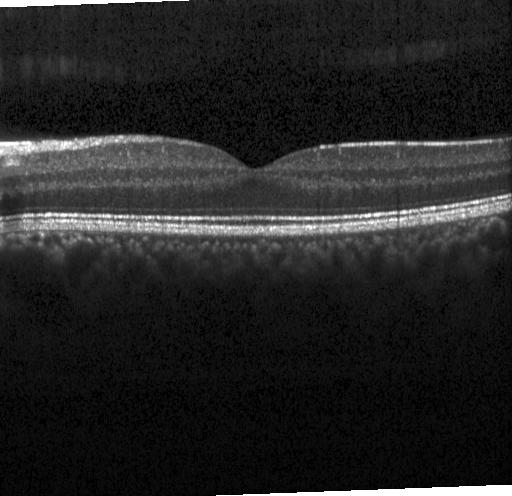 Optical coherence tomography B-scan — Finding: no choroidal neovascularization, no diabetic macular edema, and no drusen.